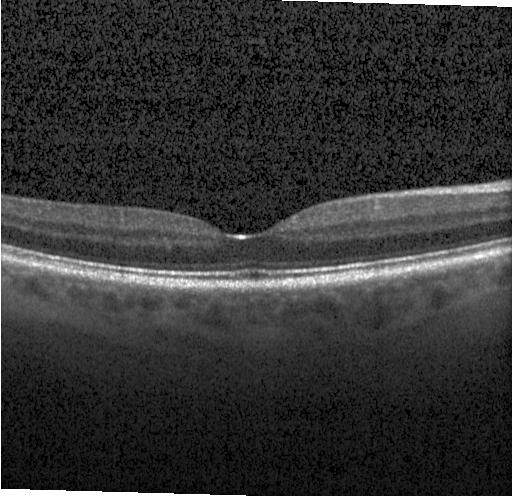

OCT B-scan showing no choroidal neovascularization, no diabetic macular edema, and no drusen.